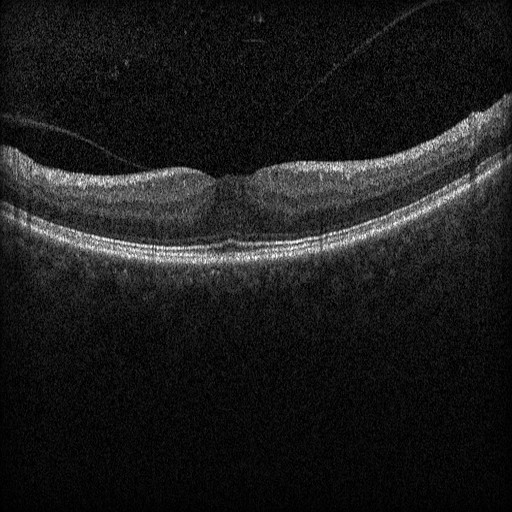

Acquired on a Heidelberg Spectralis · centered on the fovea · optical coherence tomography B-scan · spectral-domain optical coherence tomography.
Impression: DME.